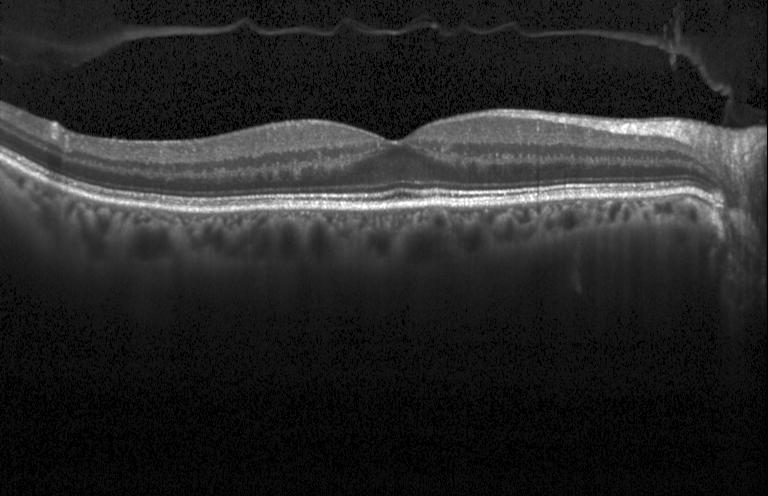

OCT finding: neither choroidal neovascularization, diabetic macular edema, nor drusen.